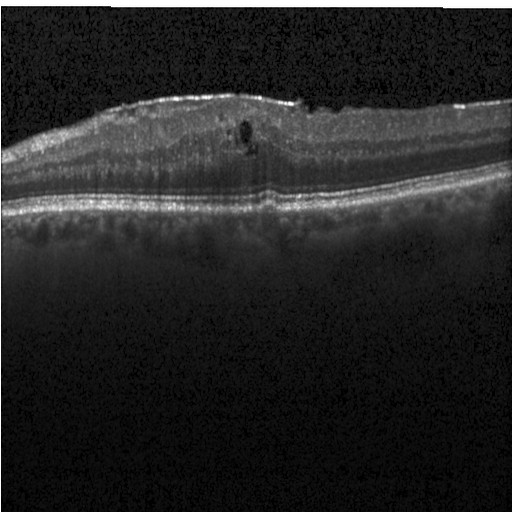

Retinal OCT B-scan; spectral-domain OCT — The scan shows diabetic macular edema (DME).